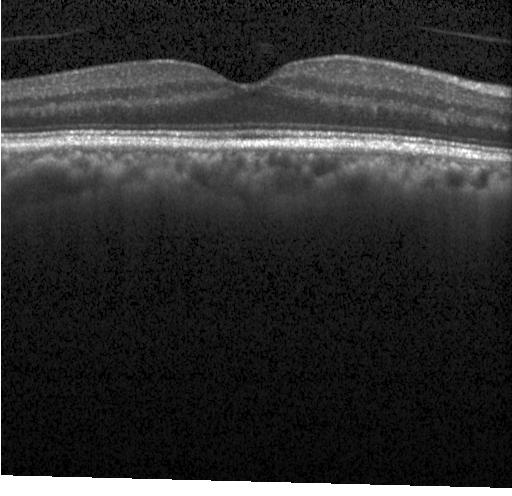
OCT line scan
Impression: no evidence of choroidal neovascularization, diabetic macular edema, or drusen.